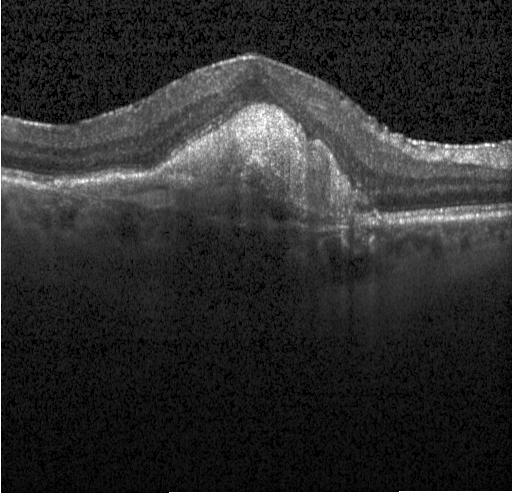 Diagnosis: a choroidal neovascular membrane.